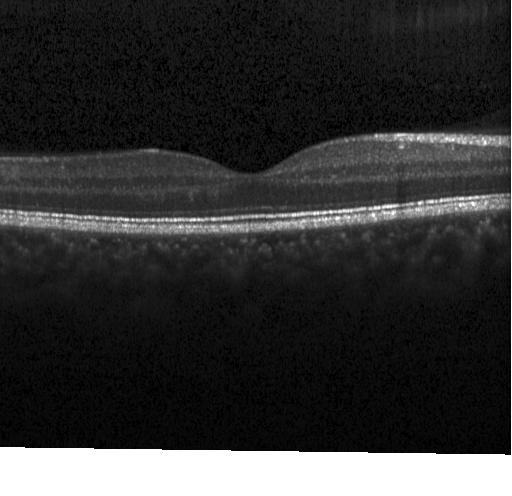 Optical coherence tomography B-scan · Heidelberg Spectralis · through the macula
Assessment: no choroidal neovascularization, diabetic macular edema, or drusen.